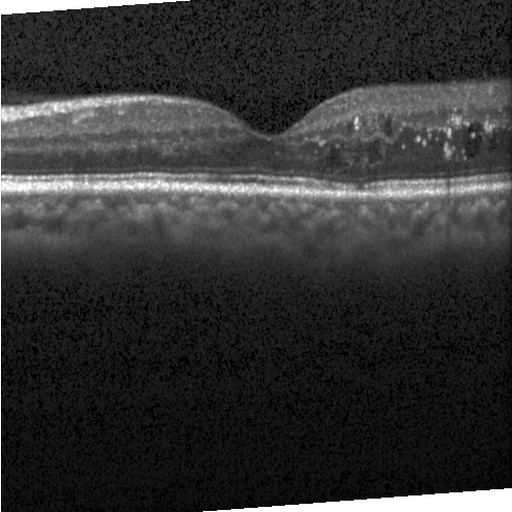 Macular scan, instrument: Heidelberg Spectralis, SD-OCT, OCT line scan. Diagnosis: DME.